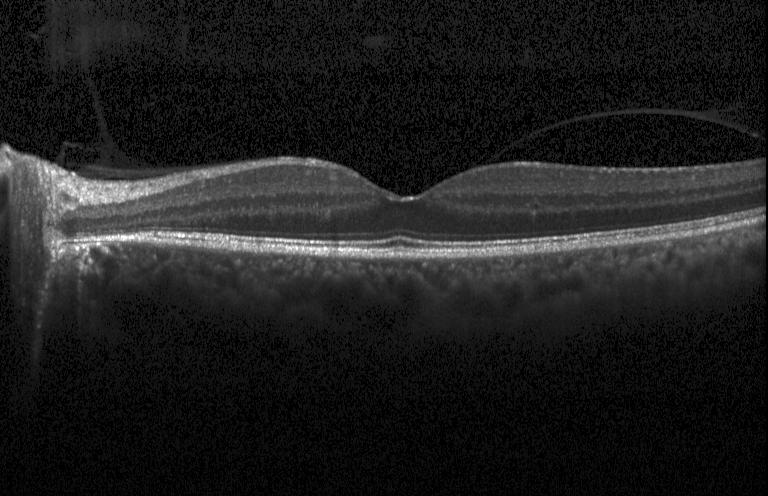 Impression: no choroidal neovascularization, no diabetic macular edema, and no drusen.